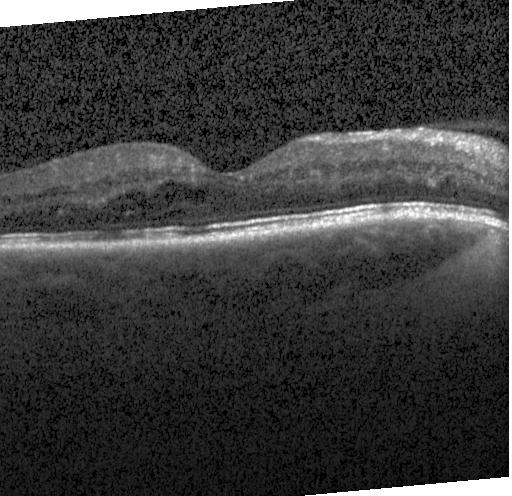

Horizontal scan through the fovea · OCT line scan · Heidelberg Spectralis · spectral-domain optical coherence tomography — The scan shows diabetic macular edema.